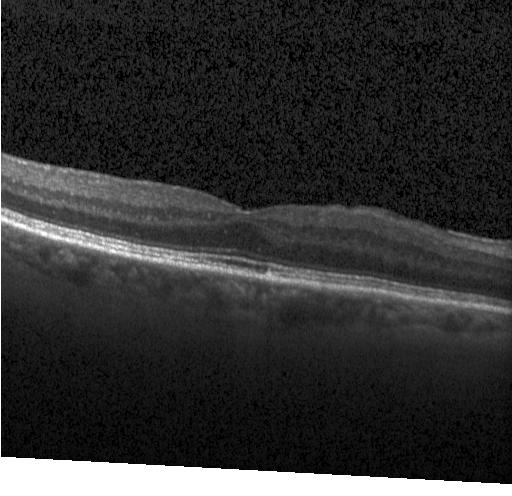
Macular scan. OCT line scan. OCT finding: no choroidal neovascularization, diabetic macular edema, or drusen.